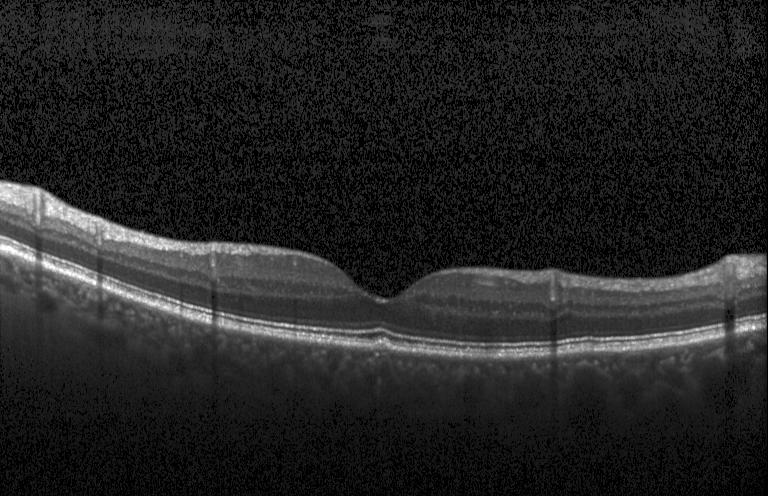

OCT finding: no choroidal neovascularization, no diabetic macular edema, and no drusen.